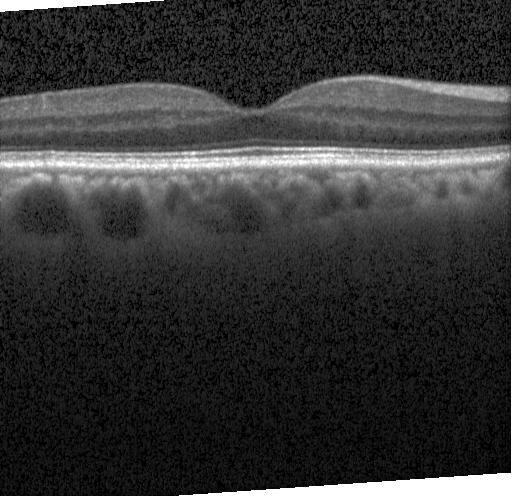 Impression: no evidence of choroidal neovascularization, diabetic macular edema, or drusen.